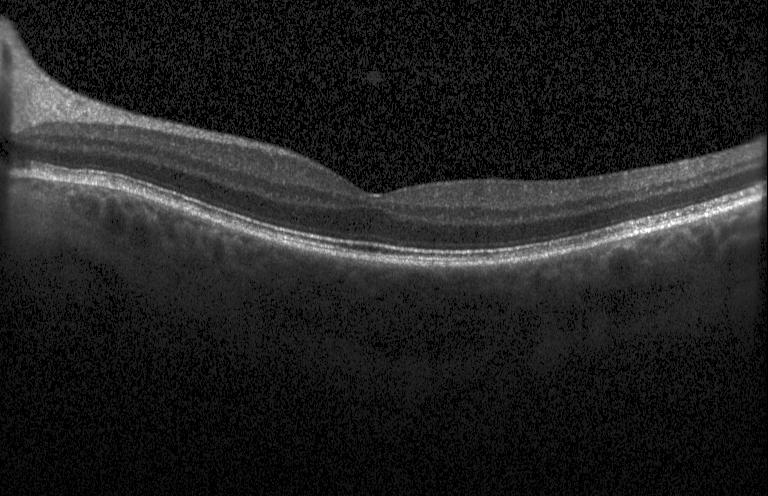 Retinal OCT B-scan. Impression: no choroidal neovascularization, diabetic macular edema, or drusen.